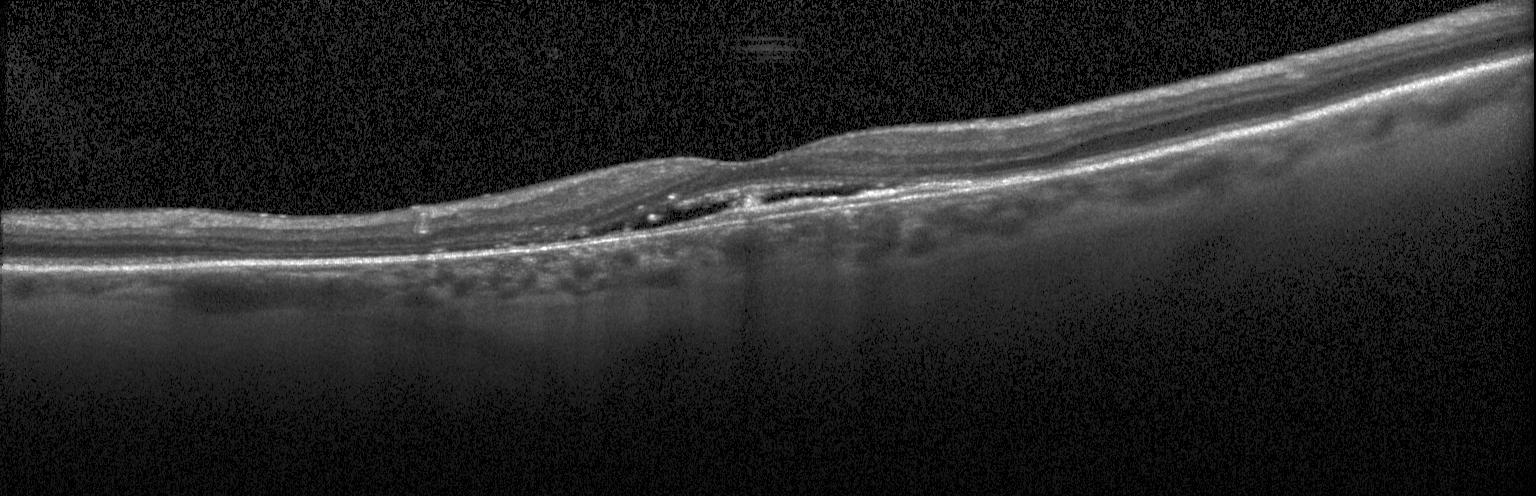
The scan shows choroidal neovascularization.